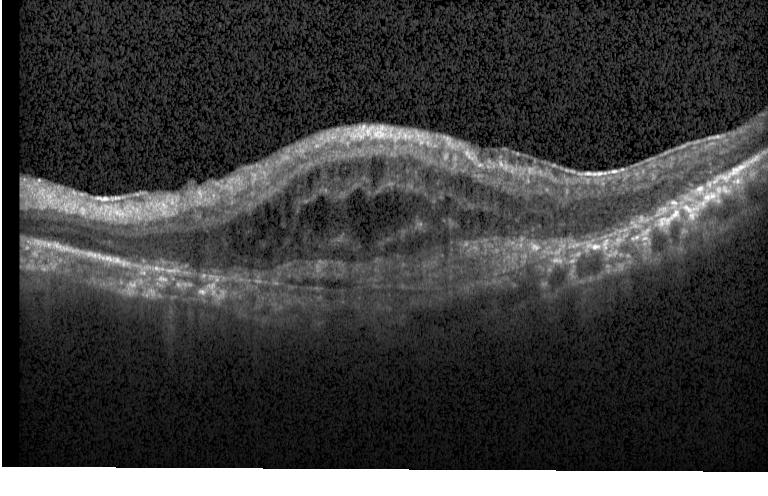 Centered on the fovea. Optical coherence tomography scan
Dx: CNV.